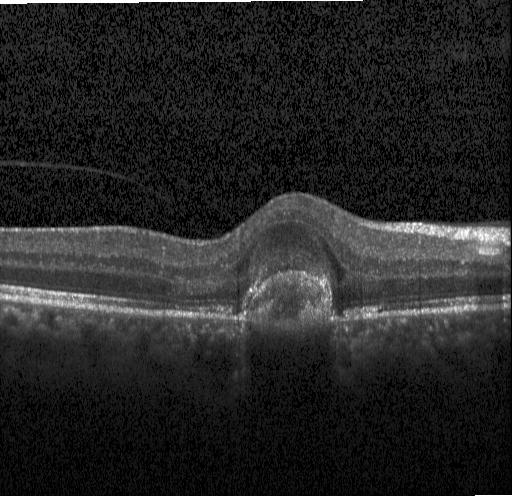
Centered on the fovea. Retinal OCT cross-section.
Assessment: a choroidal neovascular membrane.